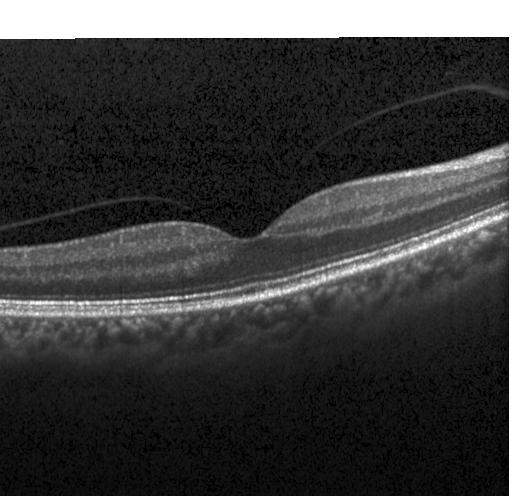

Retinal OCT cross-section showing neither CNV, DME, nor drusen.